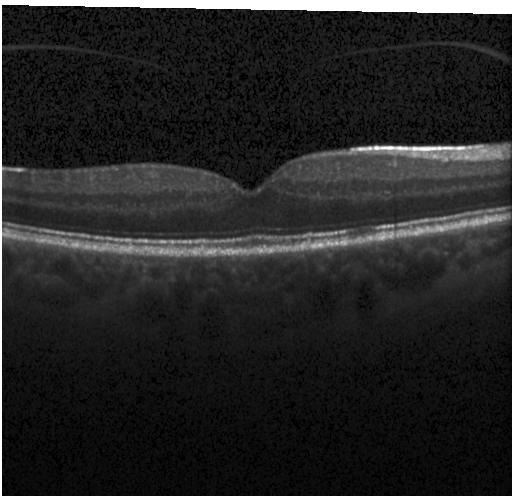
Retinal OCT B-scan, centered on the fovea, Heidelberg Spectralis OCT system, SD-OCT — Dx: neither CNV, DME, nor drusen.